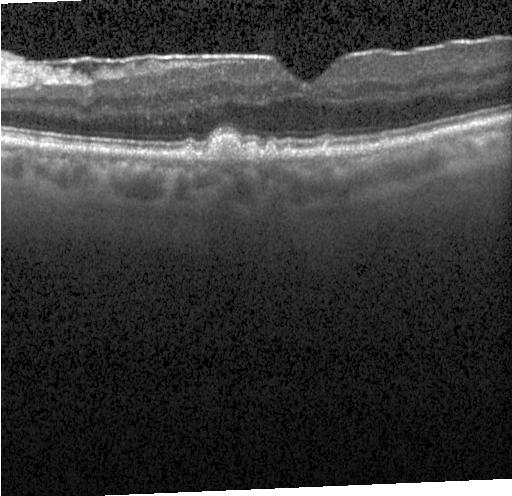 Retinal OCT B-scan
Dx: drusen.